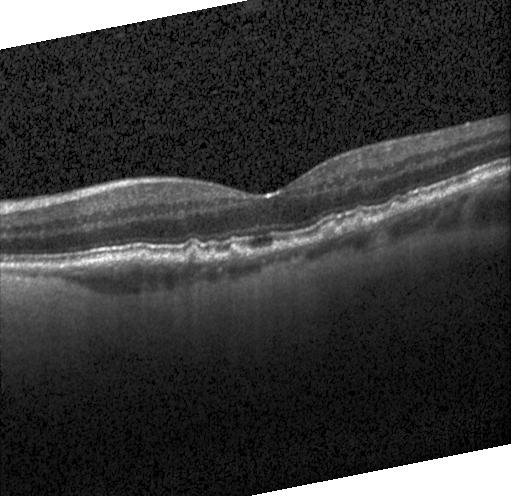

OCT B-scan showing sub-RPE drusenoid deposits.